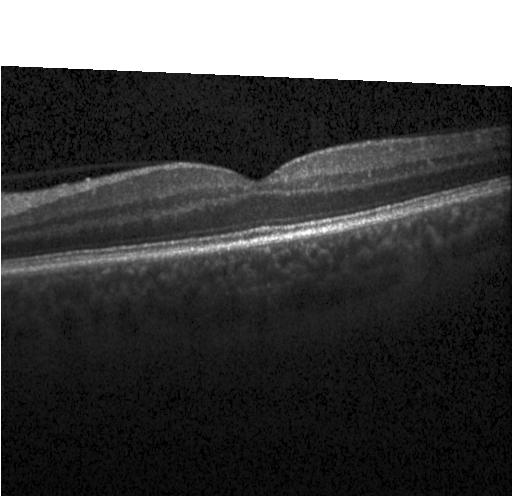 OCT line scan · centered on the fovea · Heidelberg Spectralis OCT system. The scan shows no evidence of CNV, DME, or drusen.